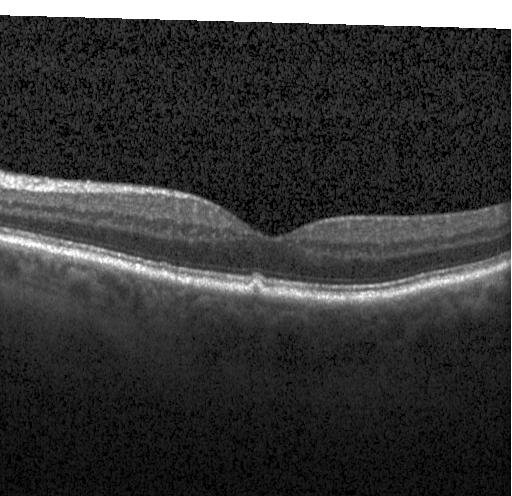

Impression: drusen.